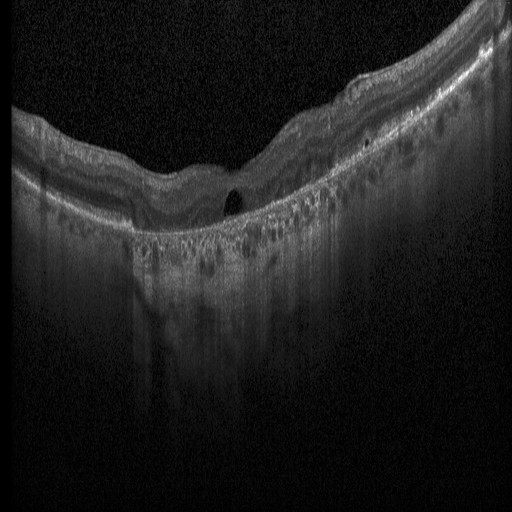
Optical coherence tomography B-scan. Diabetic macular edema.